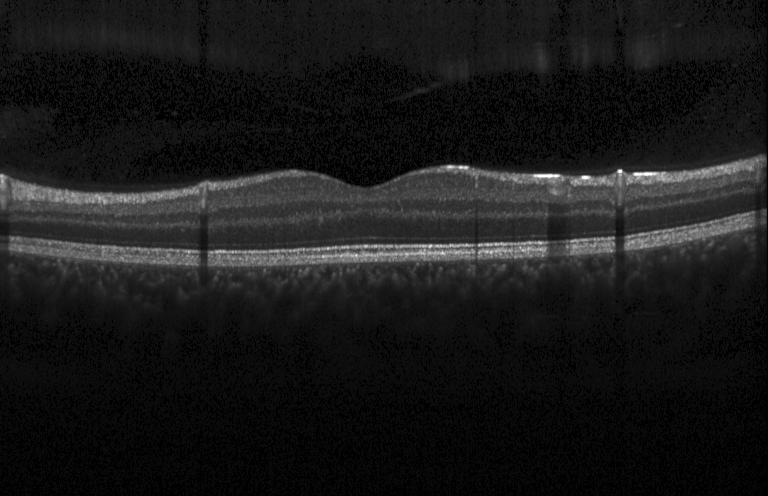 Assessment: no choroidal neovascularization, diabetic macular edema, or drusen.